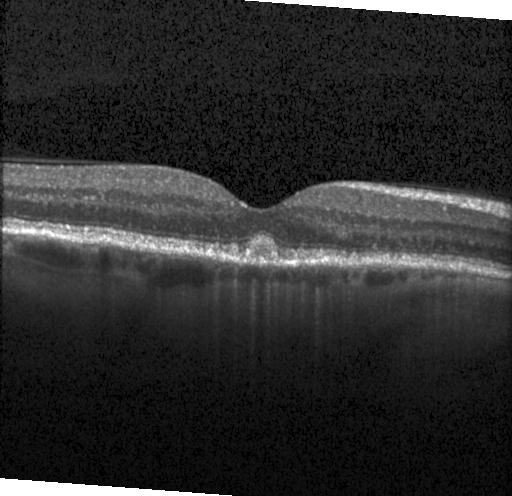
Sub-RPE drusenoid deposits.